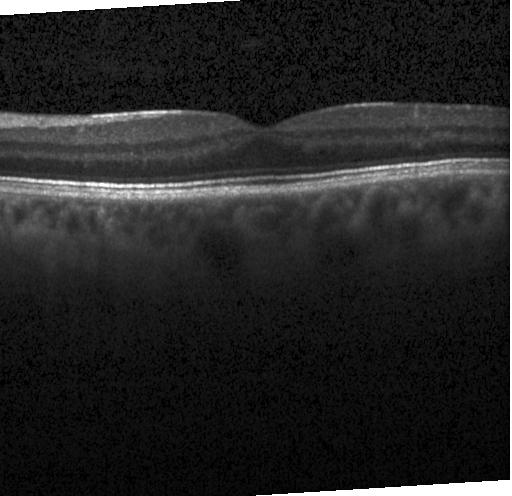
Retinal OCT B-scan — This B-scan demonstrates no choroidal neovascularization, no diabetic macular edema, and no drusen.